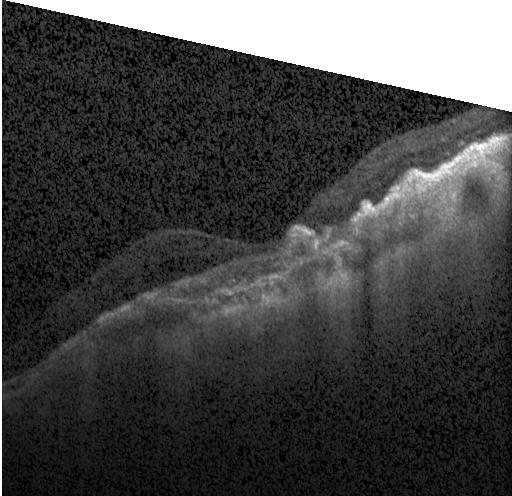

Optical coherence tomography B-scan, horizontal scan through the fovea, spectral-domain OCT, acquired on a Heidelberg Spectralis. Diagnosis: choroidal neovascularization.